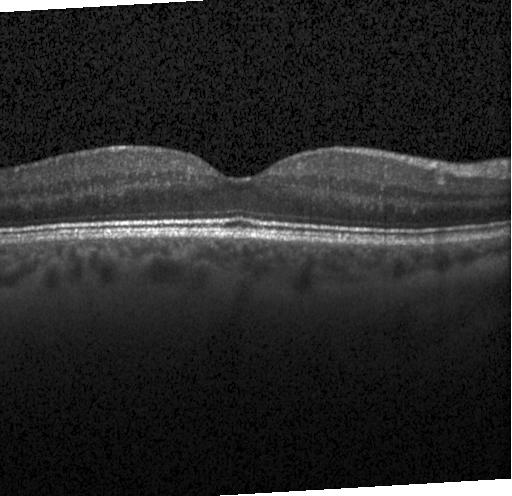 Acquired on a Heidelberg Spectralis · SD-OCT · optical coherence tomography scan. Diagnosis: neither choroidal neovascularization, diabetic macular edema, nor drusen.